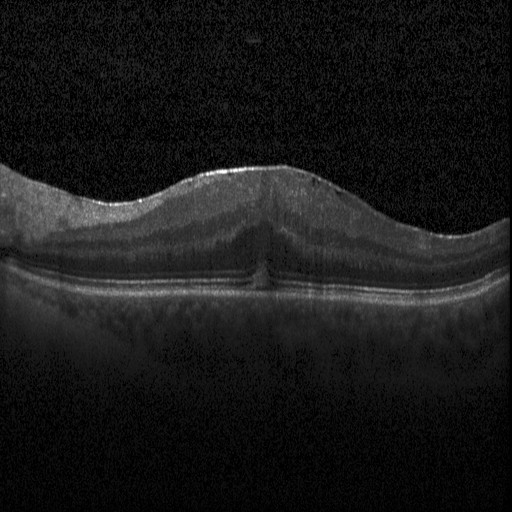 The scan shows diabetic macular edema.